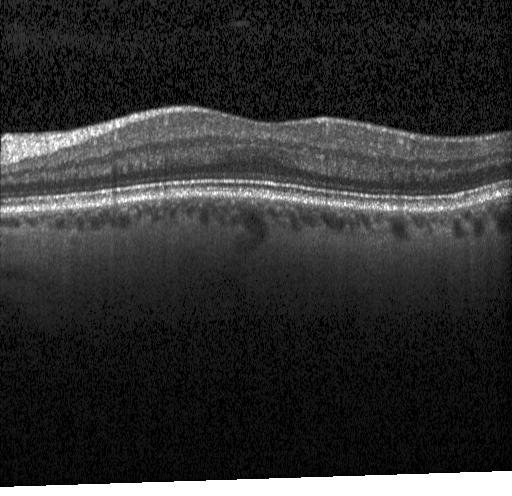 Finding: no choroidal neovascularization, diabetic macular edema, or drusen.